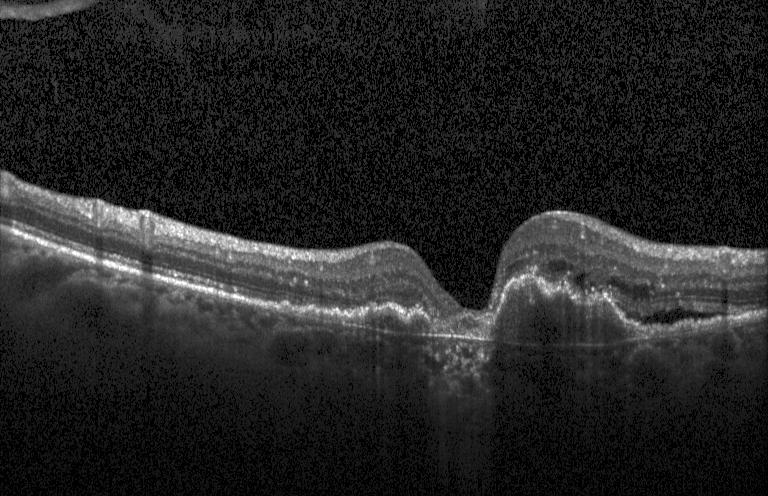
Optical coherence tomography scan — Assessment: a choroidal neovascular membrane.